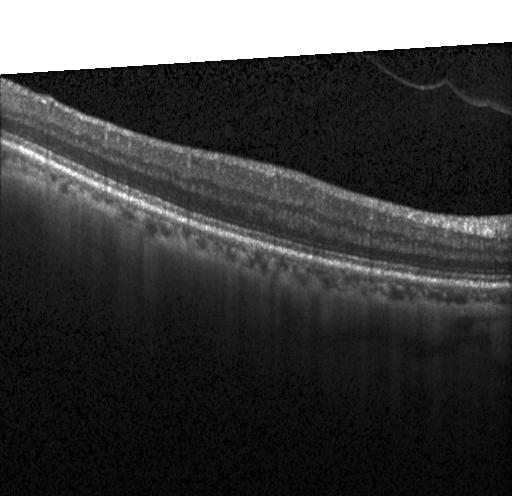 Impression: no CNV, DME, or drusen.